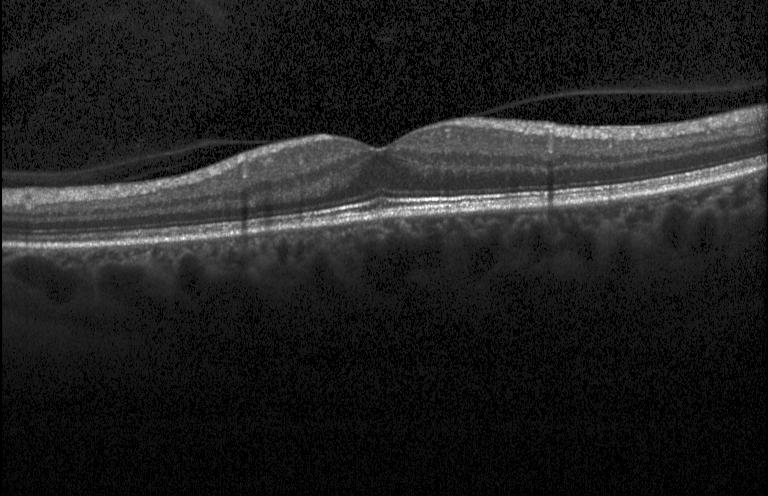 OCT B-scan; Heidelberg Spectralis; fovea-centered; SD-OCT — Impression: neither choroidal neovascularization, diabetic macular edema, nor drusen.